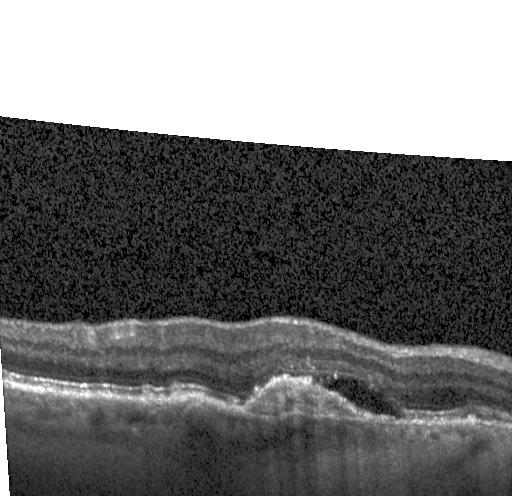

Retinal OCT cross-section · horizontal scan through the fovea · SD-OCT · acquired on a Heidelberg Spectralis — Finding: a choroidal neovascular membrane.